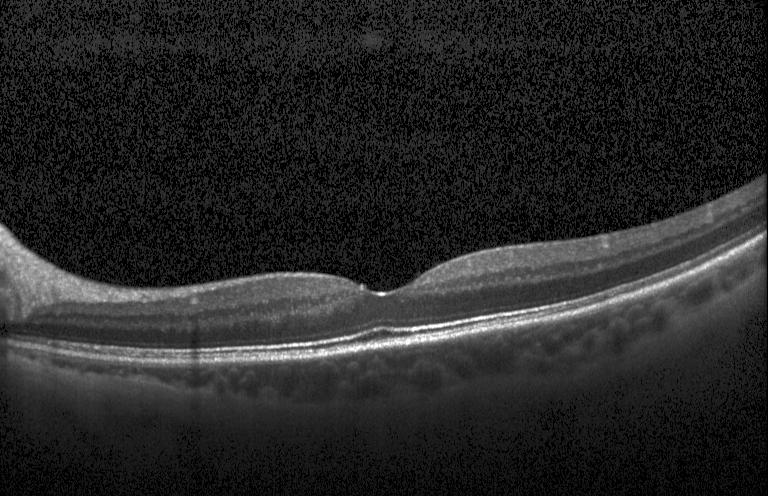

Retinal OCT cross-section showing neither CNV, DME, nor drusen.